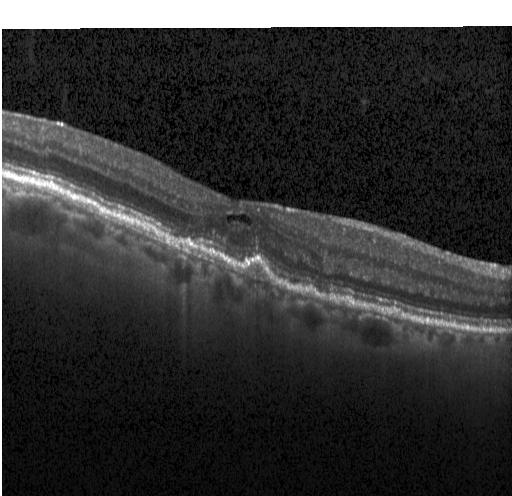
Optical coherence tomography B-scan — This B-scan demonstrates a choroidal neovascular membrane.